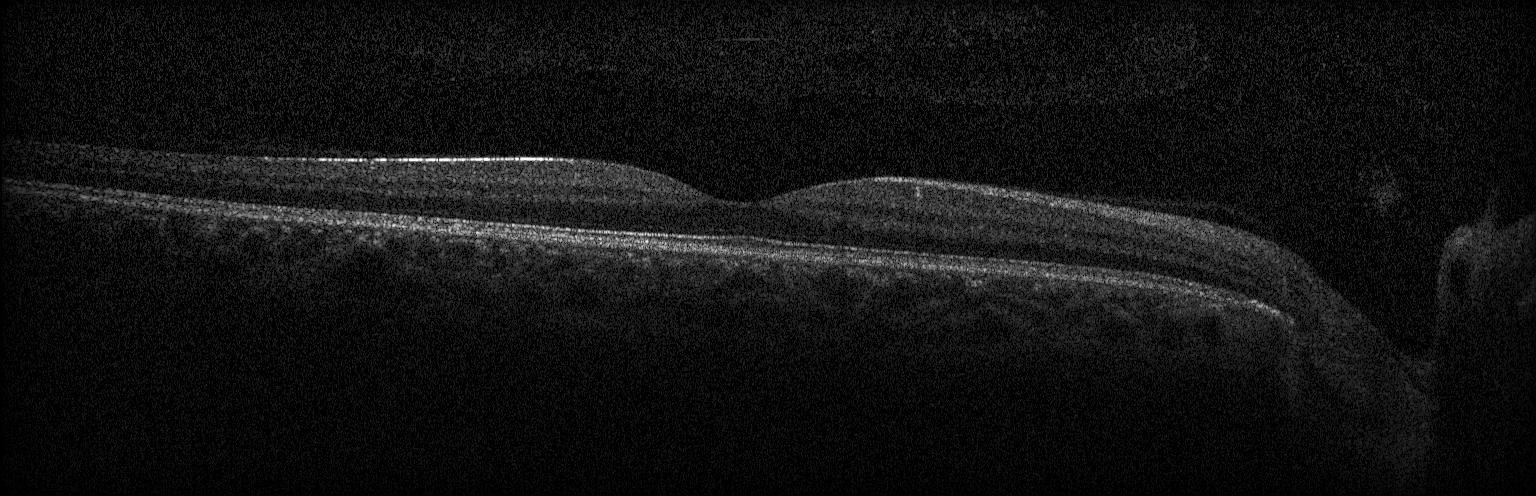

Acquired on a Heidelberg Spectralis, macular scan, optical coherence tomography scan, spectral-domain optical coherence tomography. Finding: no evidence of choroidal neovascularization, diabetic macular edema, or drusen.